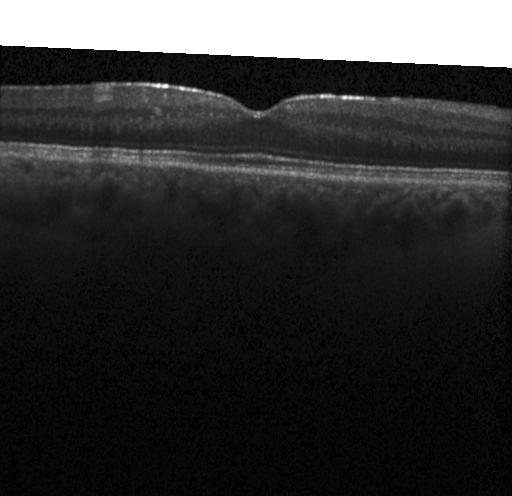

Optical coherence tomography scan.
No choroidal neovascularization, diabetic macular edema, or drusen.